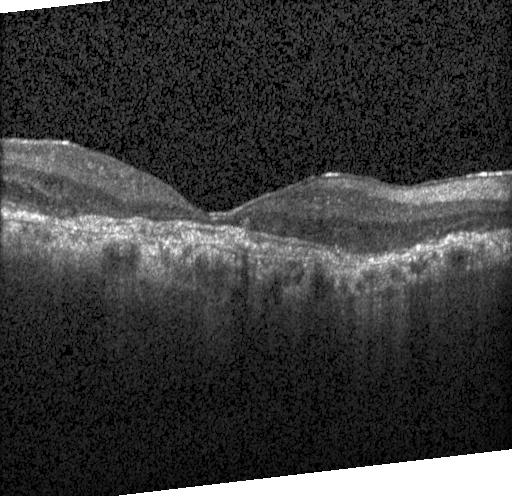 Spectral-domain OCT, horizontal scan through the fovea, retinal OCT B-scan, Heidelberg Spectralis OCT system — A choroidal neovascular membrane.